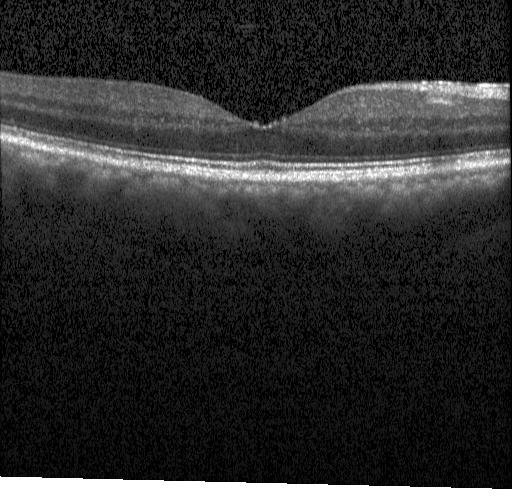 OCT B-scan showing no choroidal neovascularization, no diabetic macular edema, and no drusen.